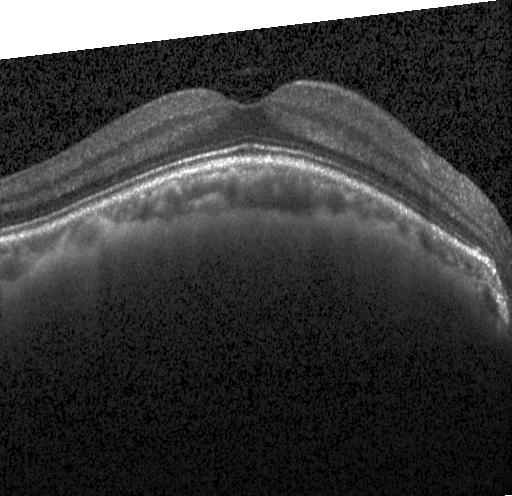 Retinal OCT B-scan.
Impression: no choroidal neovascularization, no diabetic macular edema, and no drusen.